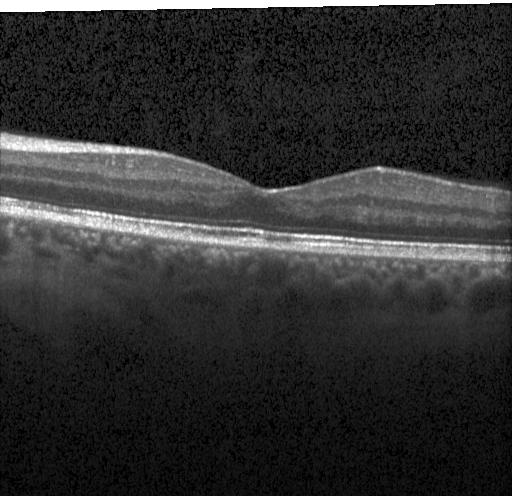

Optical coherence tomography scan; spectral-domain optical coherence tomography. Finding: no choroidal neovascularization, diabetic macular edema, or drusen.